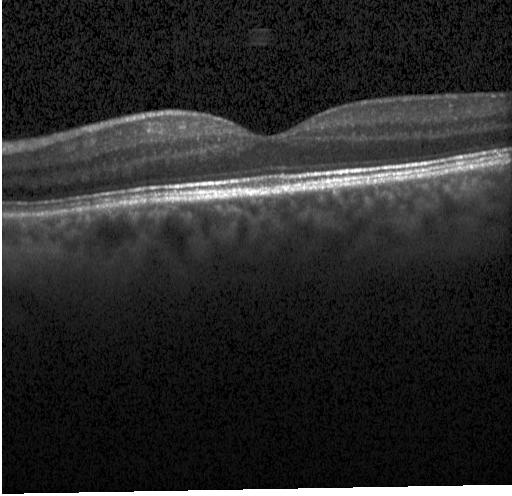

Retinal OCT cross-section · horizontal scan through the fovea · instrument: Heidelberg Spectralis · spectral-domain optical coherence tomography.
Diagnosis: no choroidal neovascularization, diabetic macular edema, or drusen.